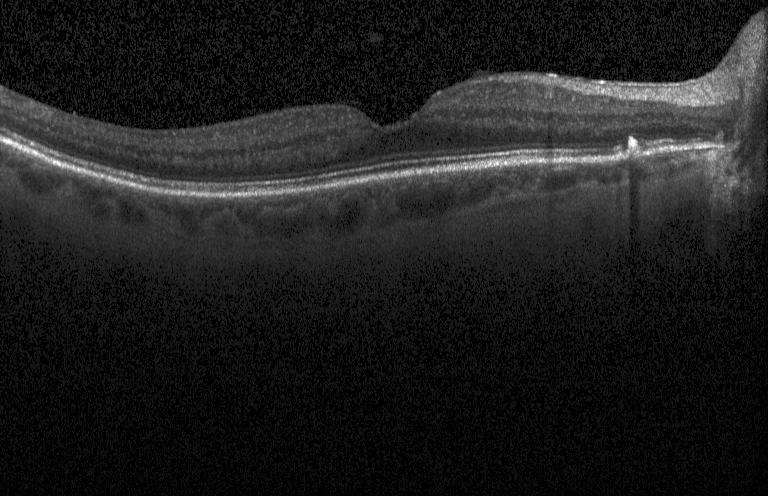

Optical coherence tomography scan — Impression: multiple drusen.